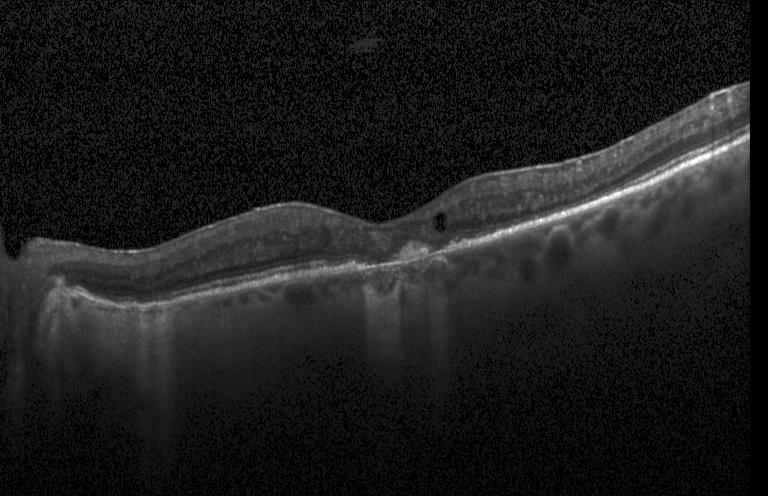

CNV.